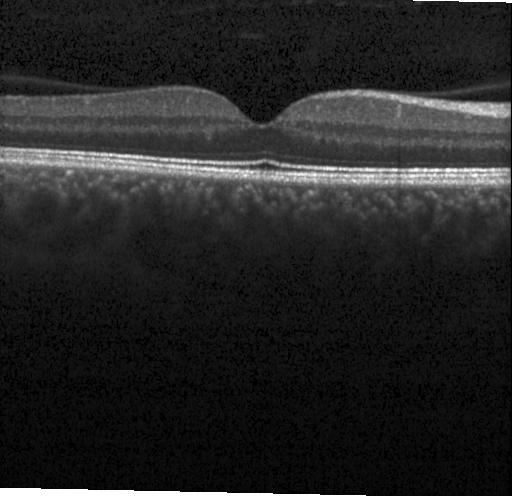
Heidelberg Spectralis · retinal OCT B-scan. No choroidal neovascularization, no diabetic macular edema, and no drusen.